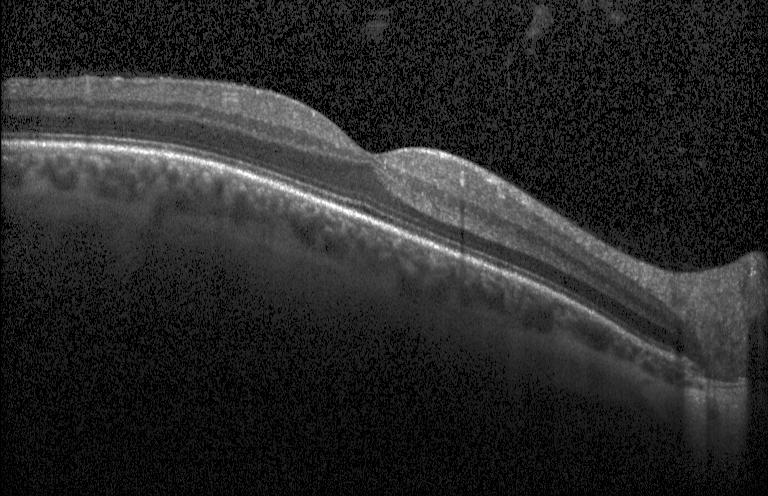
Optical coherence tomography B-scan.
Impression: no evidence of choroidal neovascularization, diabetic macular edema, or drusen.